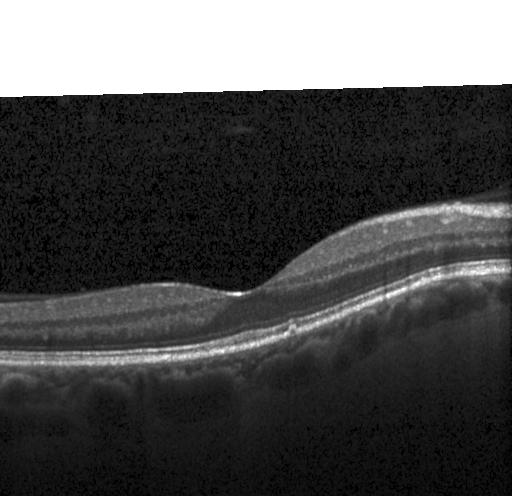
Instrument: Heidelberg Spectralis, retinal OCT cross-section. The scan shows neither choroidal neovascularization, diabetic macular edema, nor drusen.